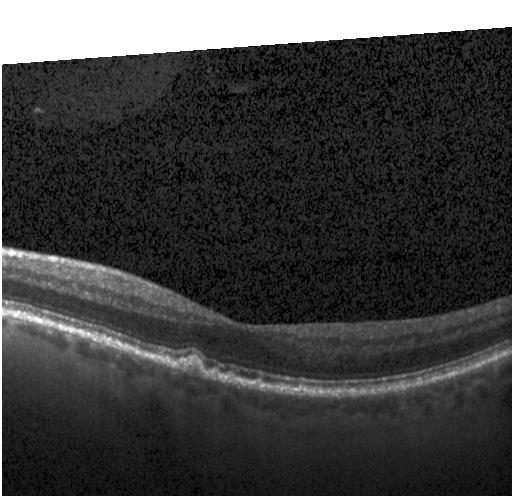 Acquired on a Heidelberg Spectralis, OCT line scan — Macular OCT: multiple drusen.